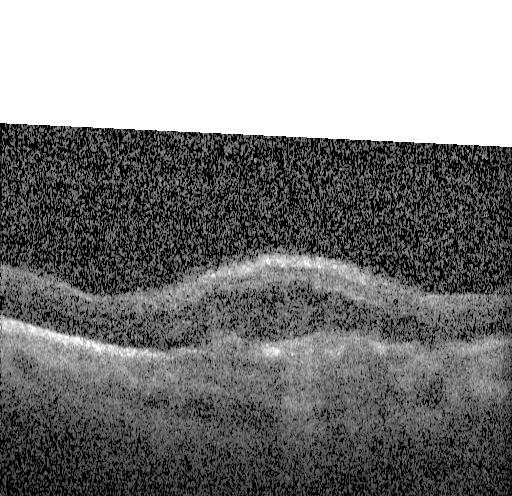 Diagnosis: a choroidal neovascular membrane.